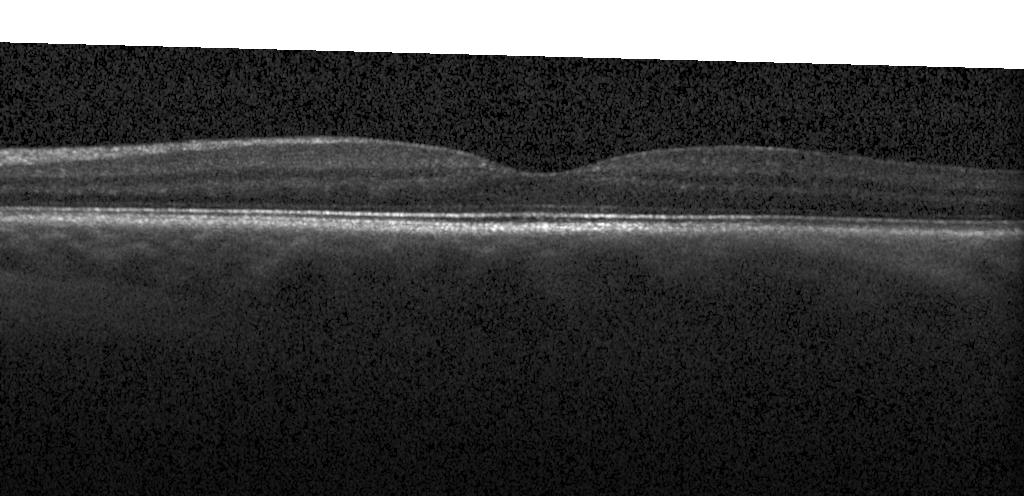 Acquired on a Heidelberg Spectralis. Optical coherence tomography scan. Spectral-domain OCT. Macular scan — Diagnosis: neither CNV, DME, nor drusen.